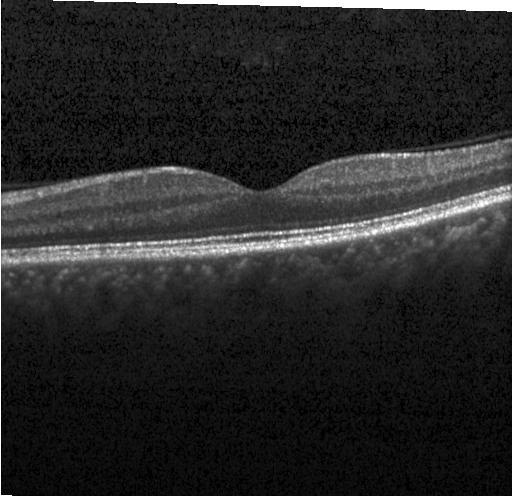
Spectral-domain OCT B-scan: no evidence of choroidal neovascularization, diabetic macular edema, or drusen.